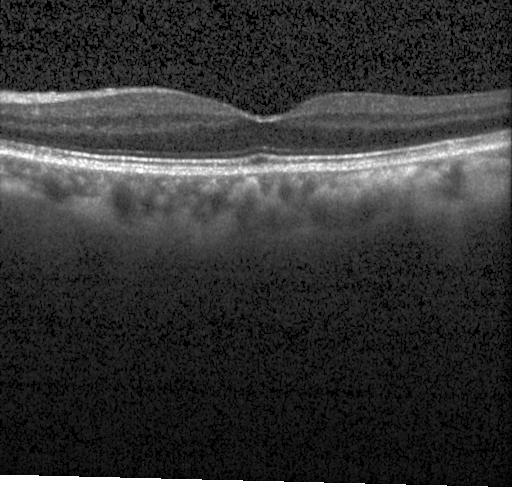 OCT scan showing neither choroidal neovascularization, diabetic macular edema, nor drusen.